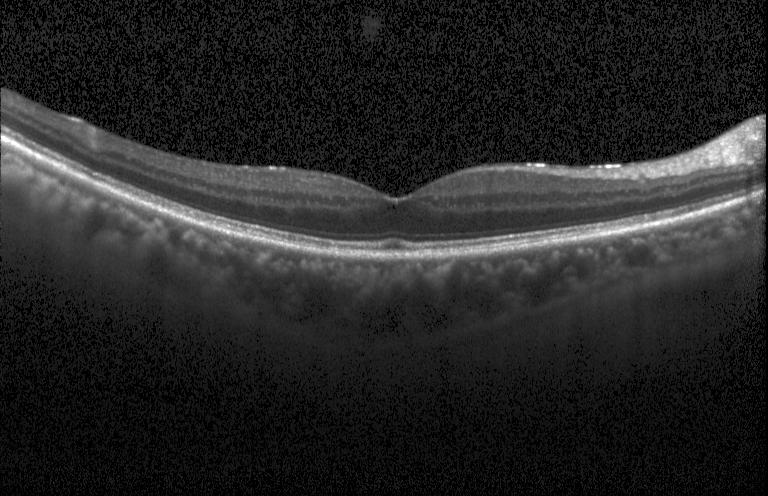

Instrument: Heidelberg Spectralis · spectral-domain optical coherence tomography · OCT B-scan — Diagnosis: no choroidal neovascularization, diabetic macular edema, or drusen.